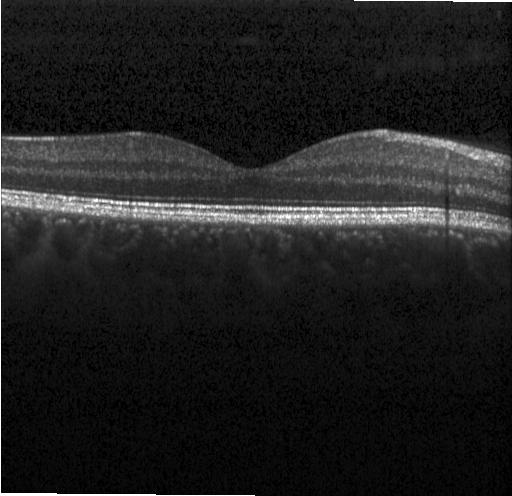
Finding: no CNV, DME, or drusen.